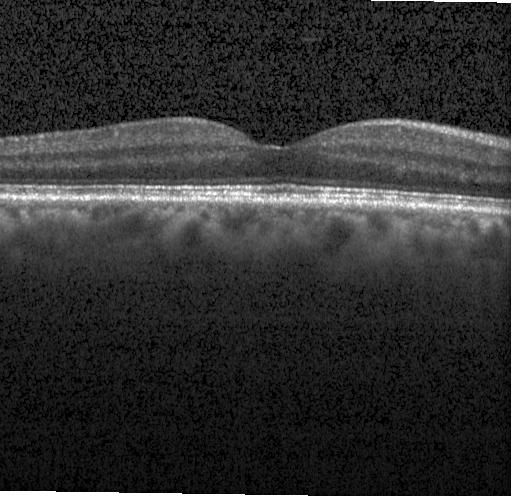
Diagnosis: no CNV, no DME, and no drusen.